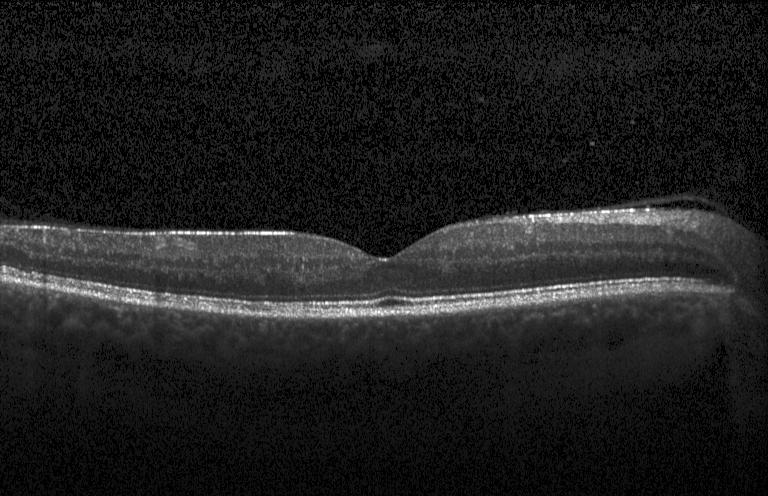

Diagnosis: no evidence of choroidal neovascularization, diabetic macular edema, or drusen.